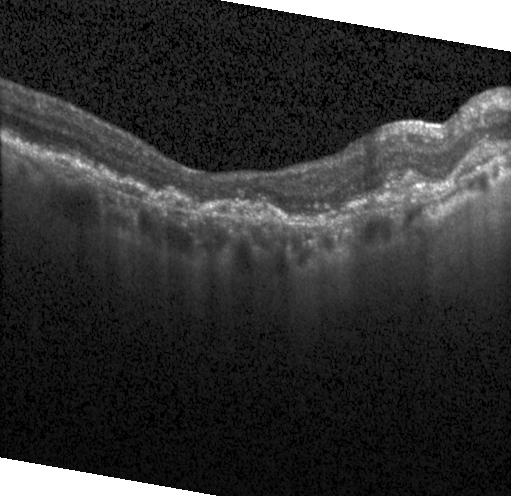

Retinal OCT cross-section showing a choroidal neovascular membrane.